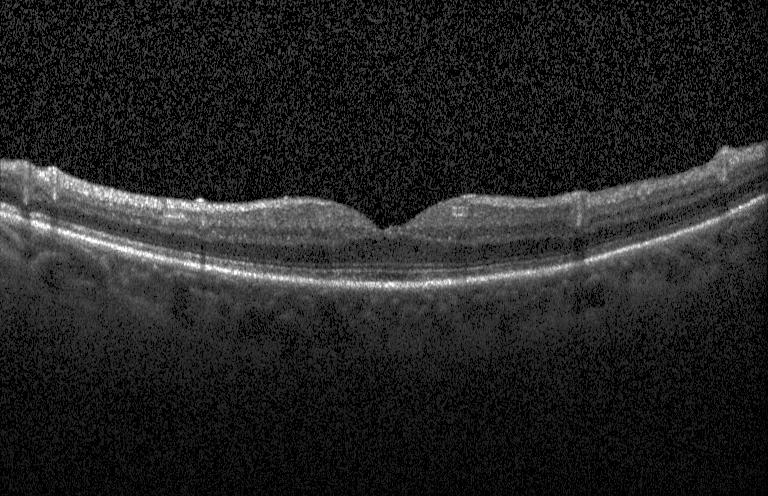

Retinal OCT cross-section showing no choroidal neovascularization, diabetic macular edema, or drusen.